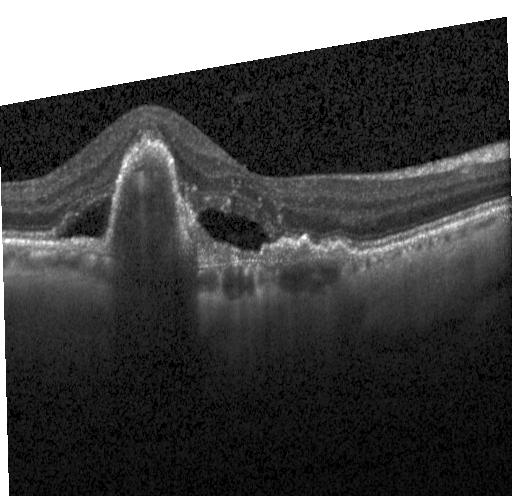 Horizontal scan through the fovea, spectral-domain optical coherence tomography, instrument: Heidelberg Spectralis, retinal OCT B-scan
Macular OCT: choroidal neovascularization.